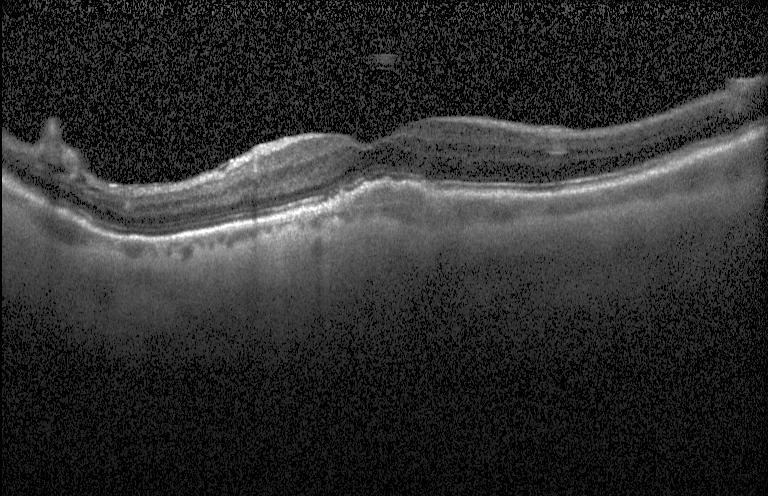
Spectral-domain optical coherence tomography. Heidelberg Spectralis OCT system. Optical coherence tomography B-scan
Impression: a choroidal neovascular membrane.